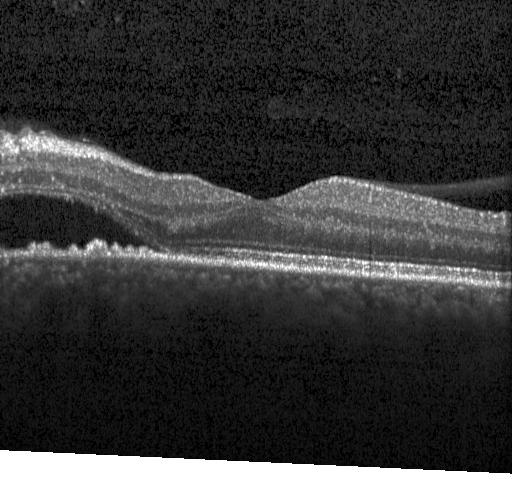 The scan shows choroidal neovascularization (CNV).